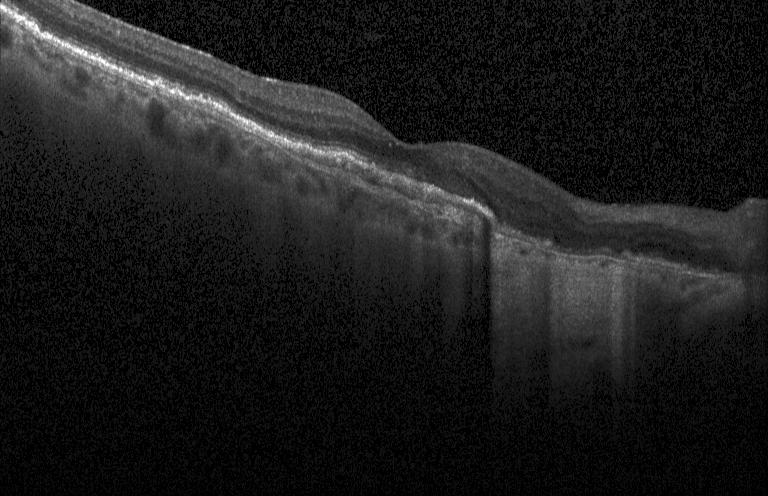

Finding: a choroidal neovascular membrane.